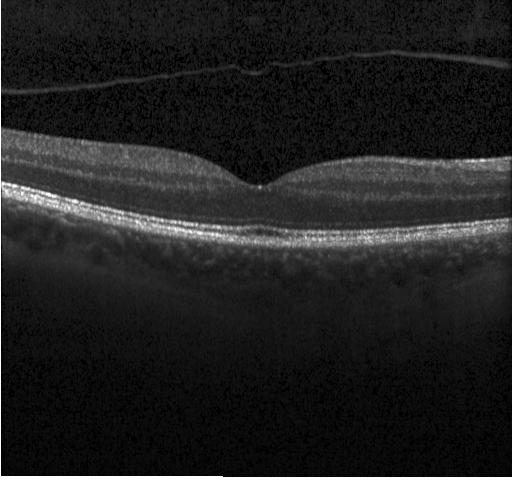

Assessment: neither choroidal neovascularization, diabetic macular edema, nor drusen.